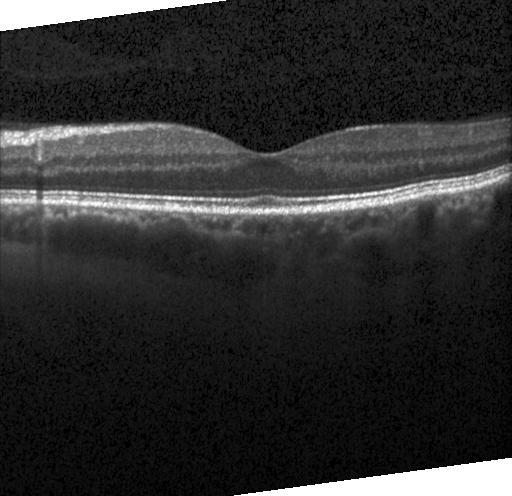 OCT line scan. Macular OCT: neither choroidal neovascularization, diabetic macular edema, nor drusen.